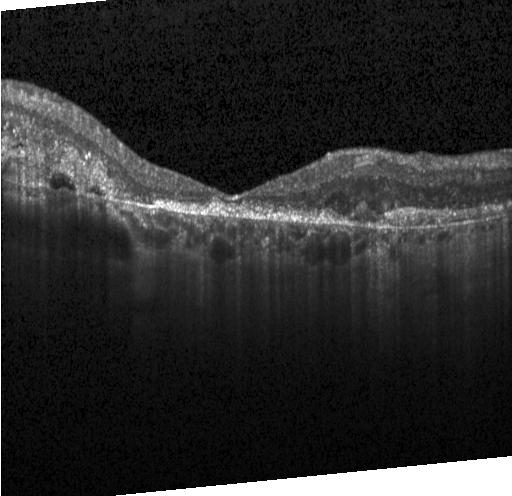
SD-OCT. Heidelberg Spectralis. Retinal OCT B-scan
Finding: a choroidal neovascular membrane.